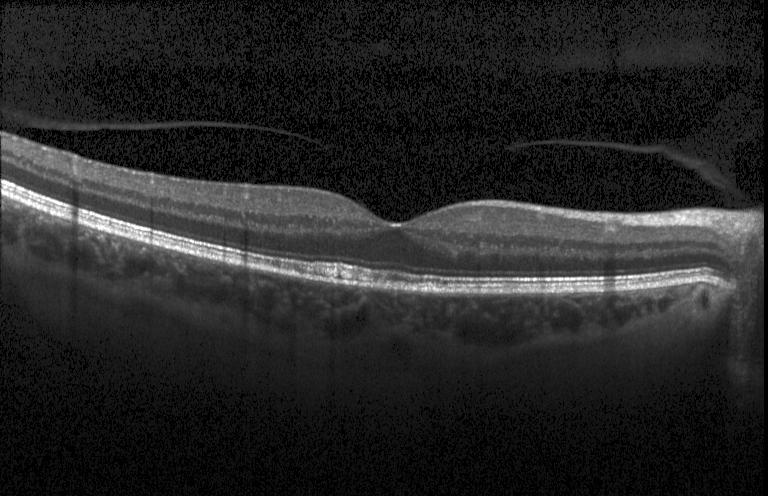 Spectral-domain OCT; retinal OCT cross-section; centered on the fovea. Finding: no choroidal neovascularization, no diabetic macular edema, and no drusen.